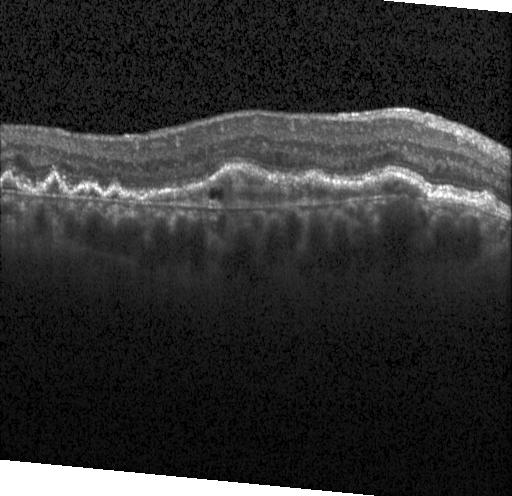 Dx: CNV.